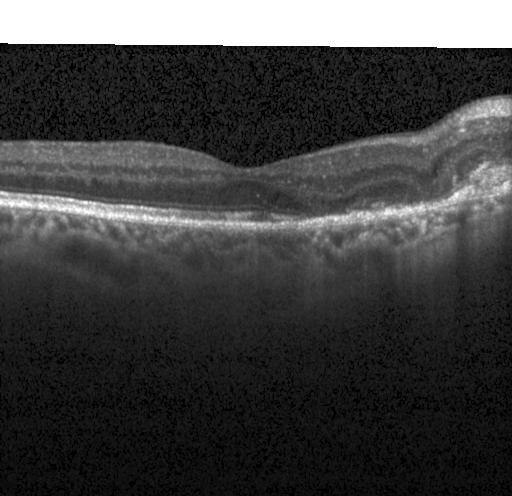
Impression: choroidal neovascularization (CNV).